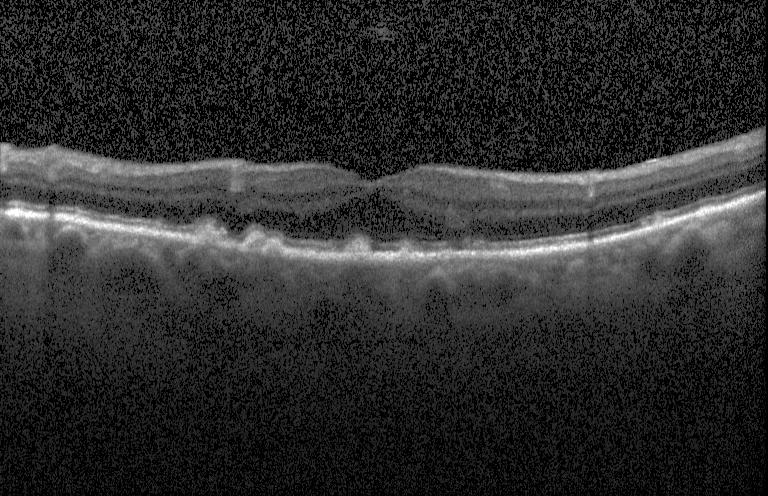 OCT line scan. Diagnosis: drusen.